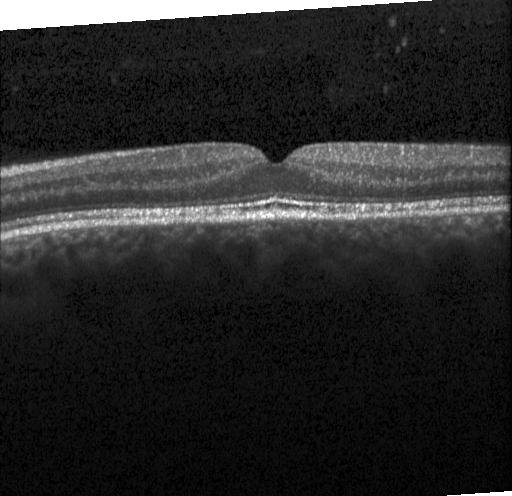 Through the macula · Heidelberg Spectralis OCT system · SD-OCT · retinal OCT cross-section. Finding: neither choroidal neovascularization, diabetic macular edema, nor drusen.